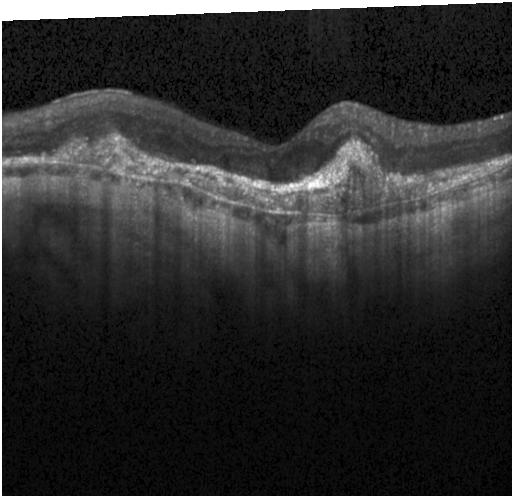 Spectral-domain OCT B-scan: a choroidal neovascular membrane.